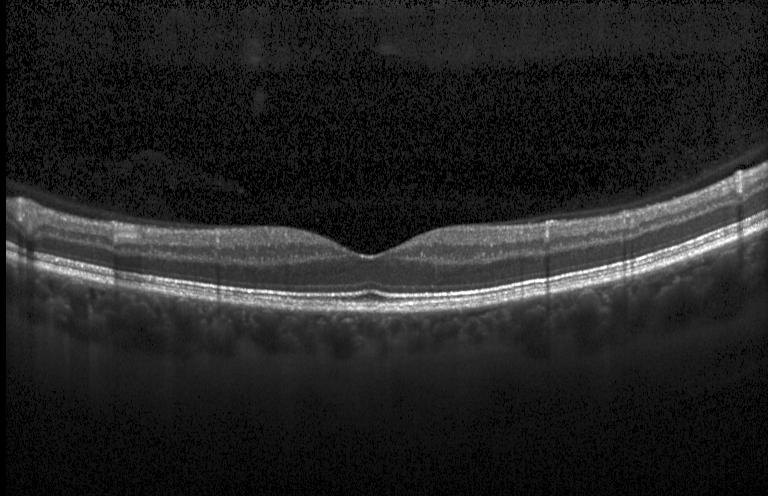 Optical coherence tomography scan. No choroidal neovascularization, diabetic macular edema, or drusen.